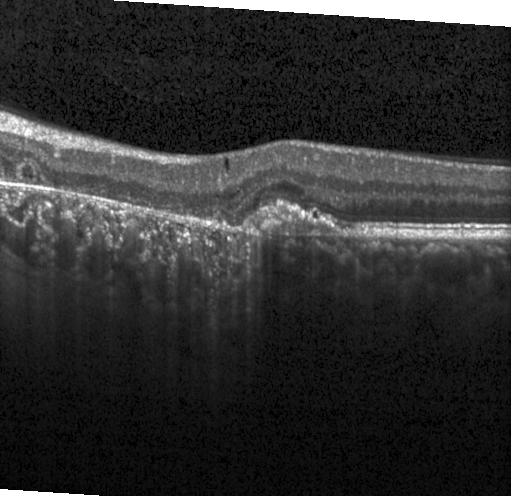

Retinal OCT B-scan. Spectral-domain OCT. This B-scan demonstrates choroidal neovascularization (CNV).